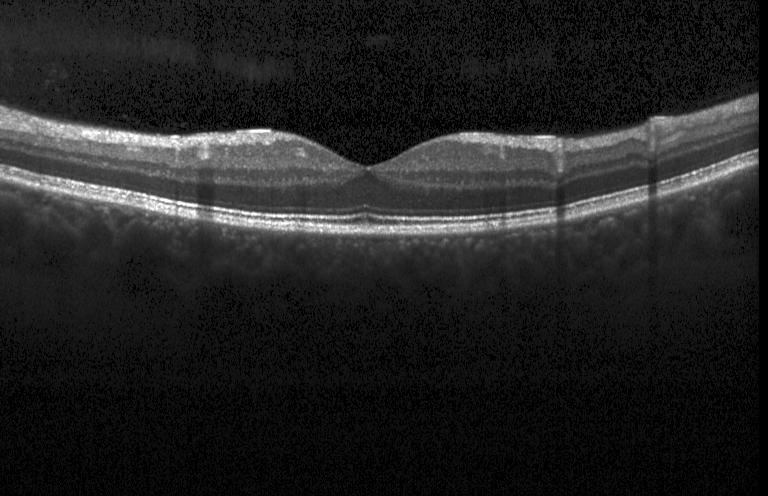
Retinal OCT cross-section; macular scan; spectral-domain OCT; acquired on a Heidelberg Spectralis
The scan shows no choroidal neovascularization, no diabetic macular edema, and no drusen.